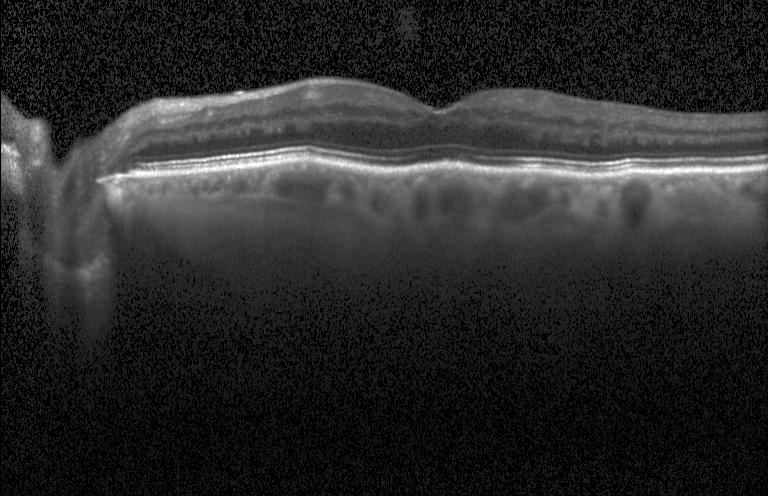
This B-scan demonstrates no choroidal neovascularization, diabetic macular edema, or drusen.